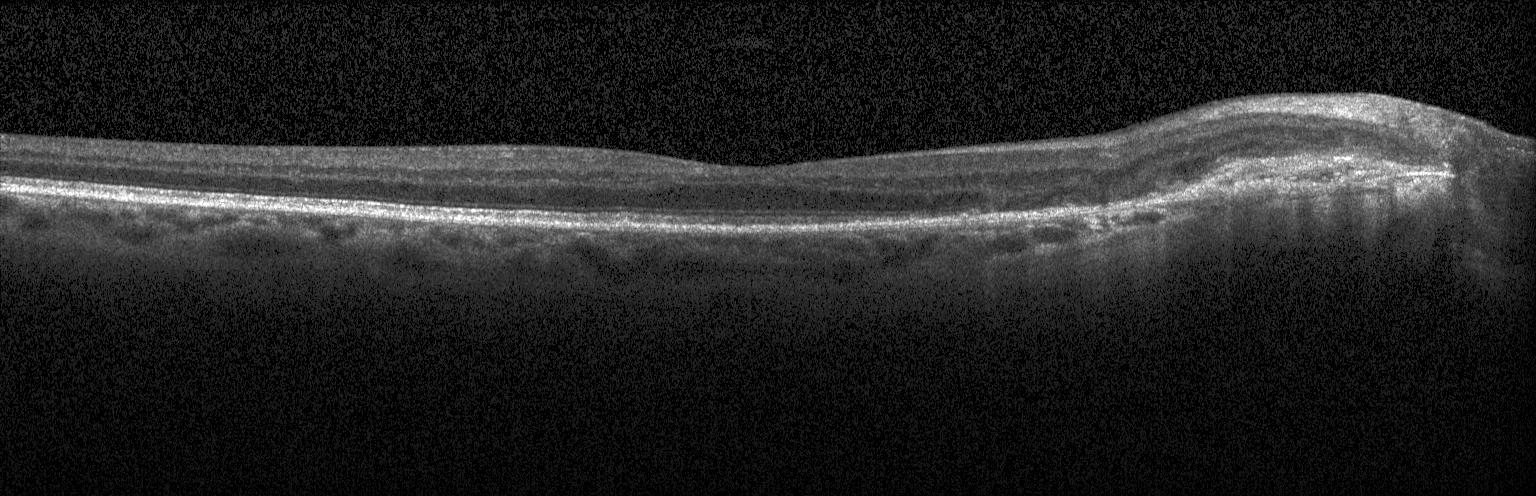
Centered on the fovea. Optical coherence tomography scan. Spectral-domain optical coherence tomography — Macular OCT: a choroidal neovascular membrane.